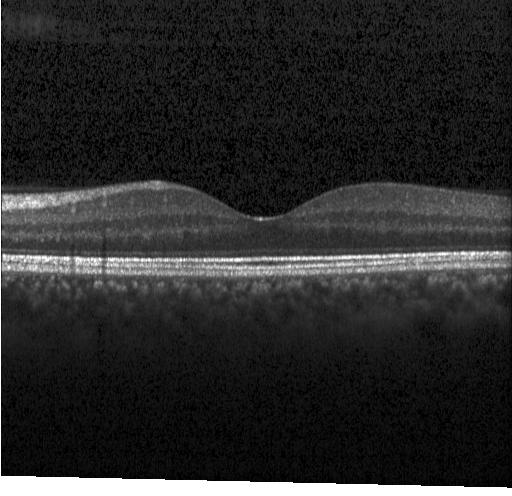
Optical coherence tomography B-scan.
Impression: neither choroidal neovascularization, diabetic macular edema, nor drusen.